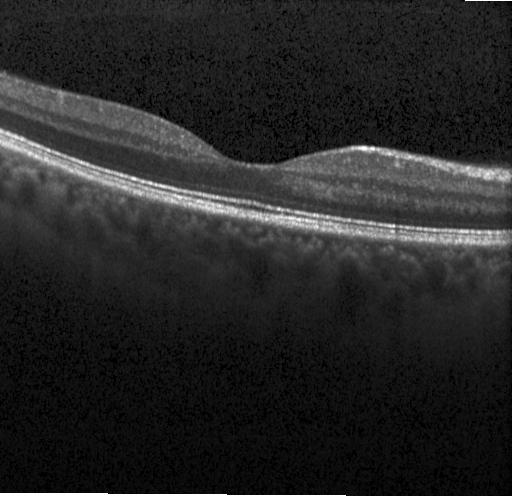
Retinal OCT cross-section. SD-OCT.
Finding: neither choroidal neovascularization, diabetic macular edema, nor drusen.